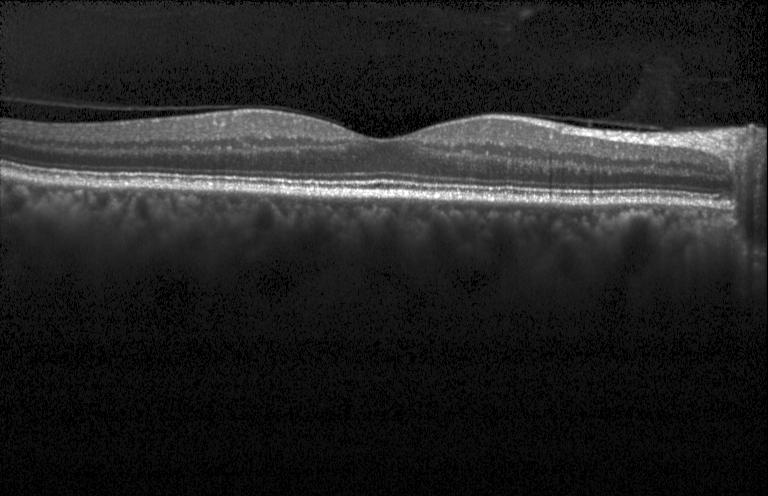 Instrument: Heidelberg Spectralis · SD-OCT · OCT B-scan — Diagnosis: neither choroidal neovascularization, diabetic macular edema, nor drusen.